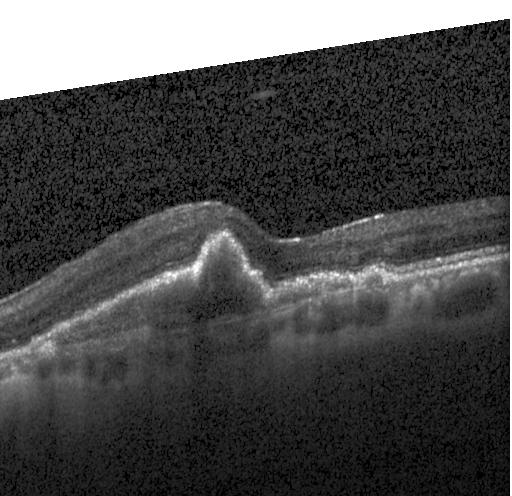 Optical coherence tomography scan · through the macula · Heidelberg Spectralis OCT system. Finding: a choroidal neovascular membrane.